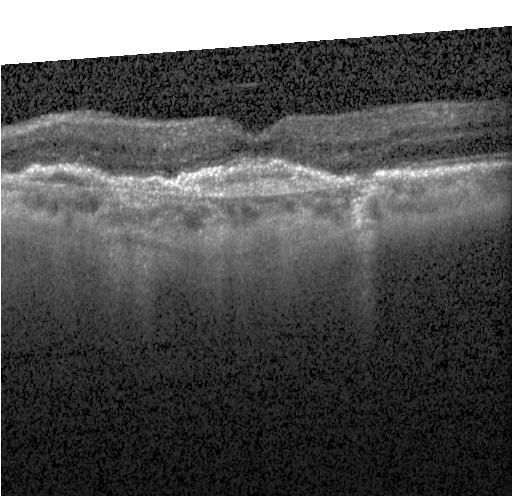 Optical coherence tomography B-scan · horizontal scan through the fovea — OCT finding: choroidal neovascularization.